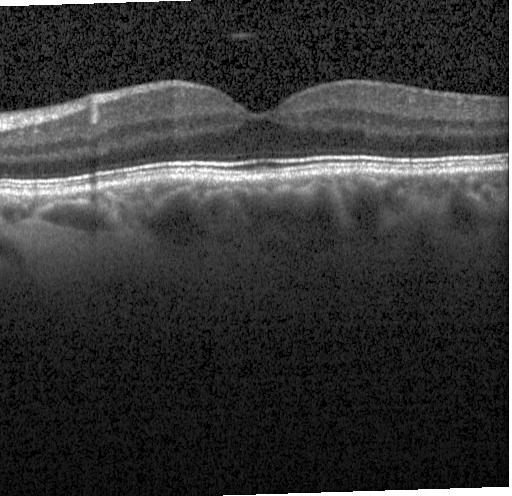
Finding: no choroidal neovascularization, no diabetic macular edema, and no drusen.